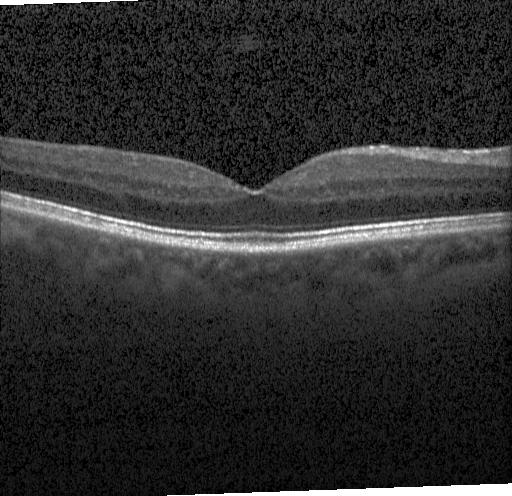
Optical coherence tomography scan, horizontal scan through the fovea, Heidelberg Spectralis.
This B-scan demonstrates neither choroidal neovascularization, diabetic macular edema, nor drusen.